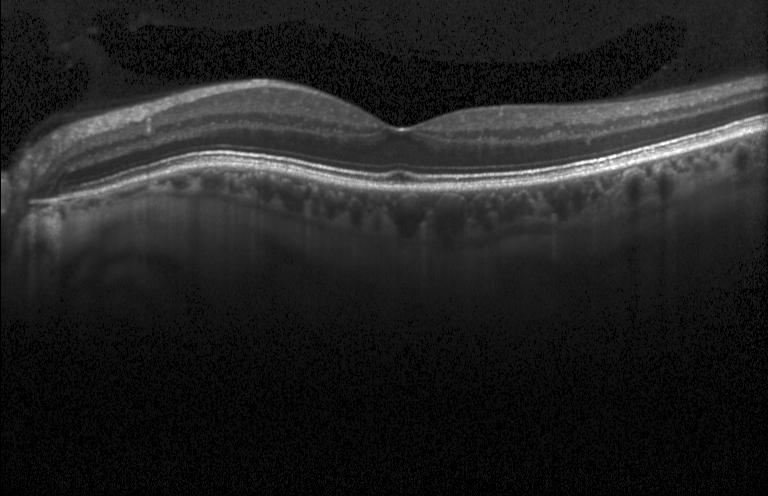 Diagnosis: no choroidal neovascularization, no diabetic macular edema, and no drusen.